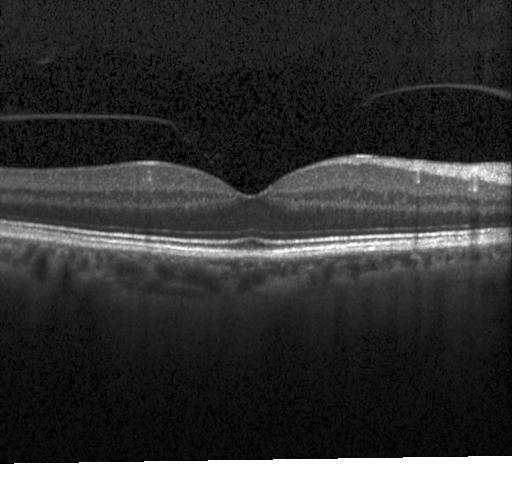 Dx: no choroidal neovascularization, diabetic macular edema, or drusen.